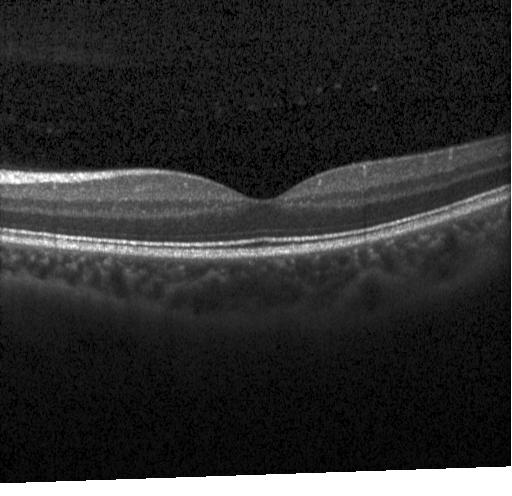 Macular OCT demonstrating no choroidal neovascularization, diabetic macular edema, or drusen.